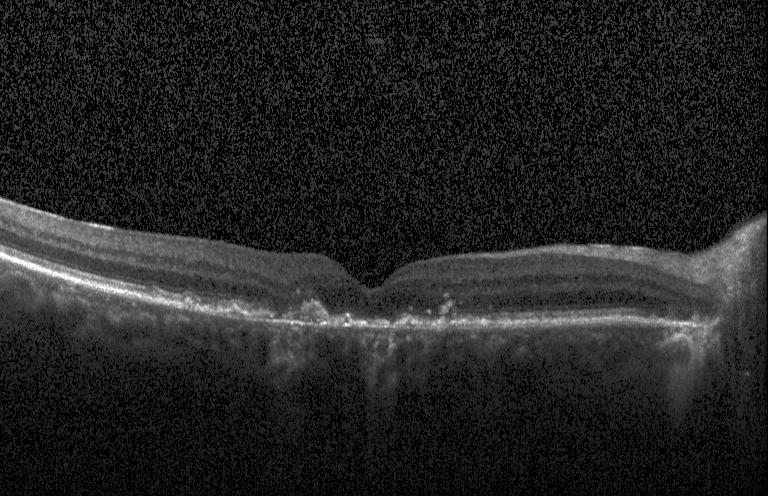
Assessment: a choroidal neovascular membrane.